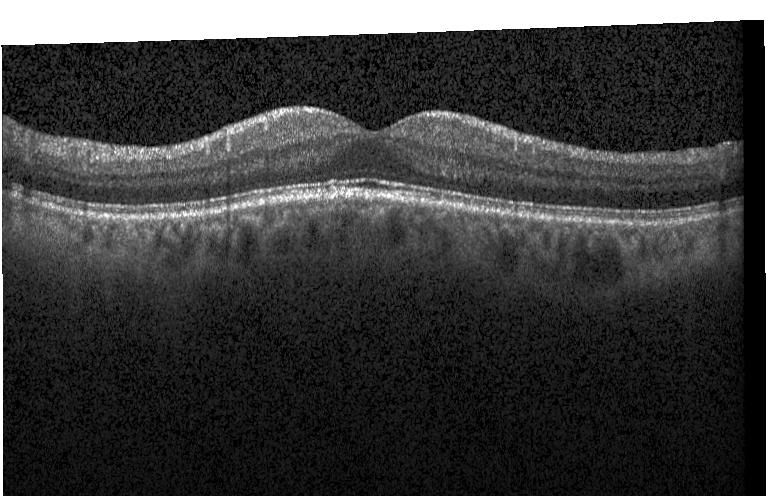

Spectral-domain OCT B-scan: no CNV, no DME, and no drusen.